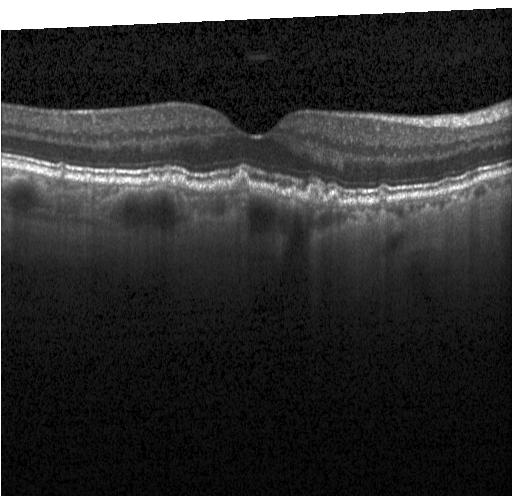
Optical coherence tomography scan · SD-OCT — Macular OCT: multiple drusen.